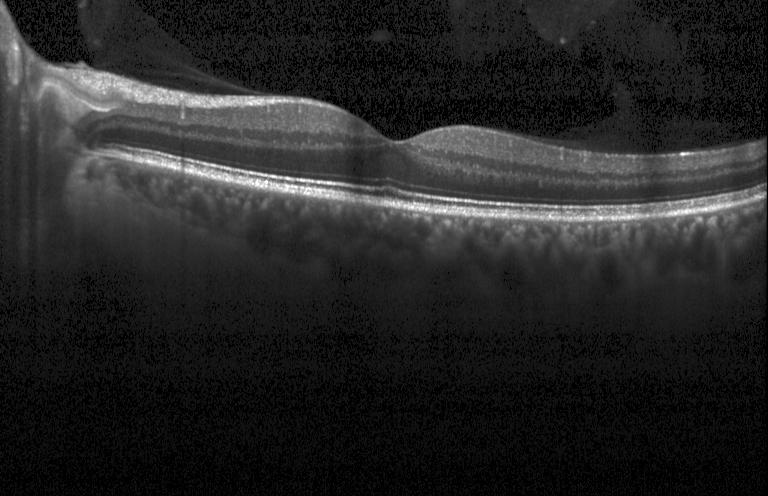 Optical coherence tomography scan.
OCT finding: no evidence of choroidal neovascularization, diabetic macular edema, or drusen.